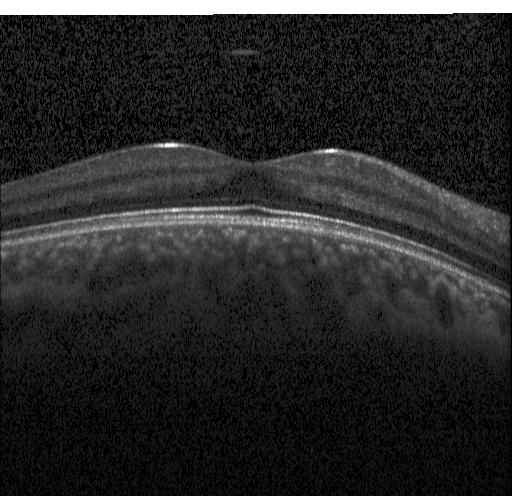 Impression: no evidence of choroidal neovascularization, diabetic macular edema, or drusen.